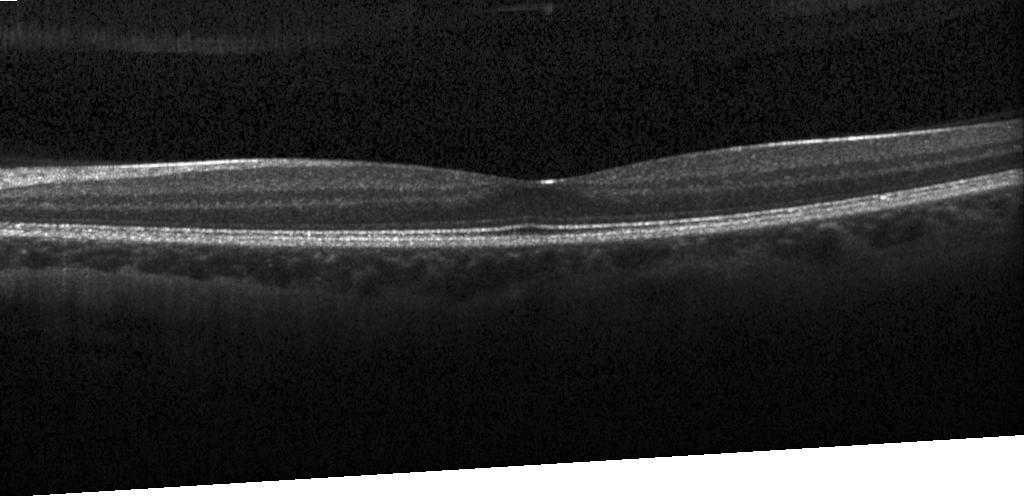
Assessment: no CNV, no DME, and no drusen.